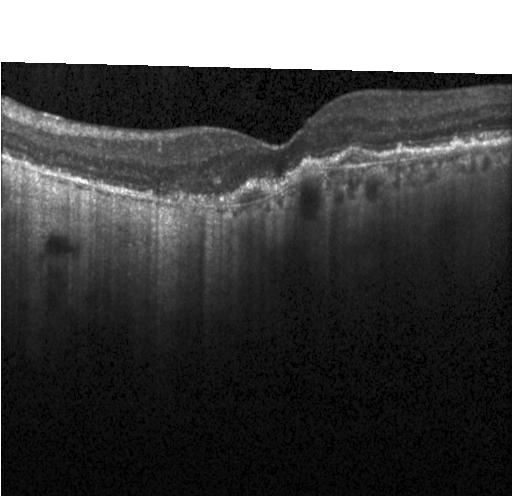

Diagnosis: CNV.